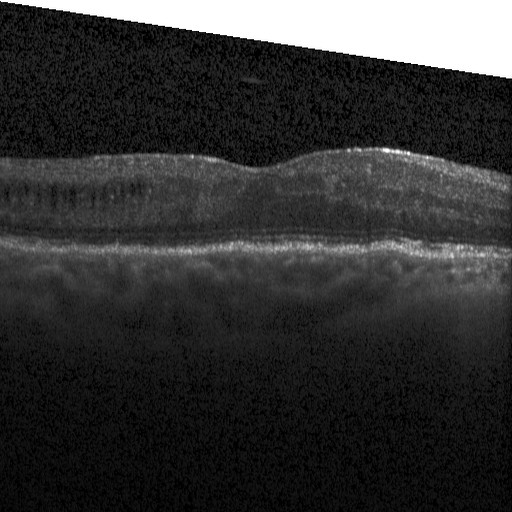
OCT line scan, instrument: Heidelberg Spectralis
This B-scan demonstrates diabetic macular edema (DME).